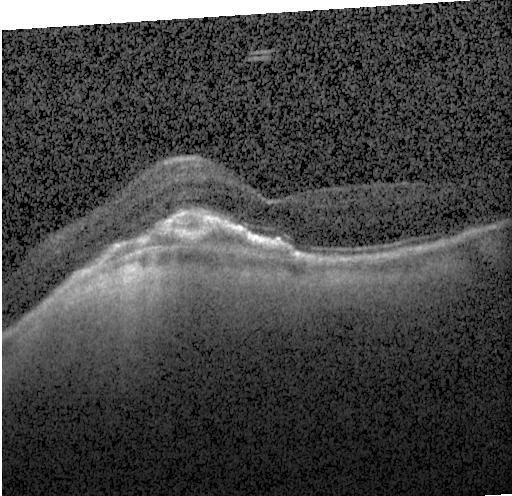

Impression: choroidal neovascularization.